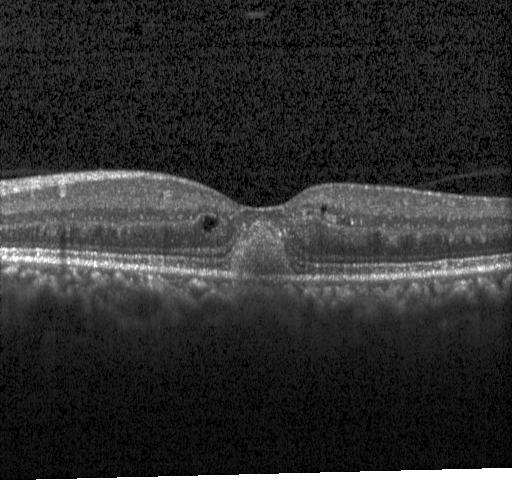
OCT B-scan
The scan shows a choroidal neovascular membrane.